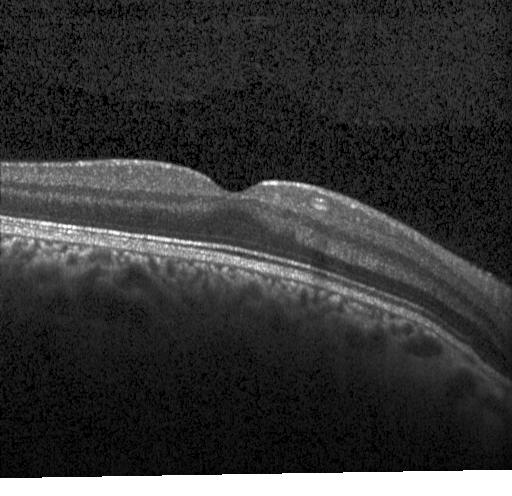

Spectral-domain optical coherence tomography. Retinal OCT B-scan. Acquired on a Heidelberg Spectralis — This B-scan demonstrates no choroidal neovascularization, no diabetic macular edema, and no drusen.